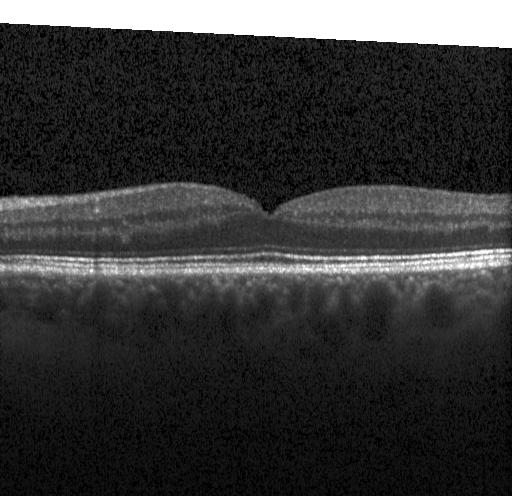
Heidelberg Spectralis; spectral-domain optical coherence tomography; retinal OCT cross-section; through the macula.
Neither CNV, DME, nor drusen.